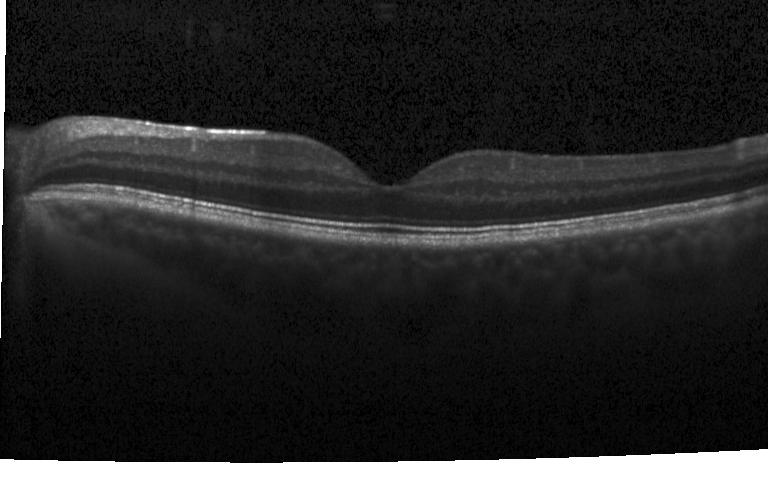

Impression: no evidence of CNV, DME, or drusen.